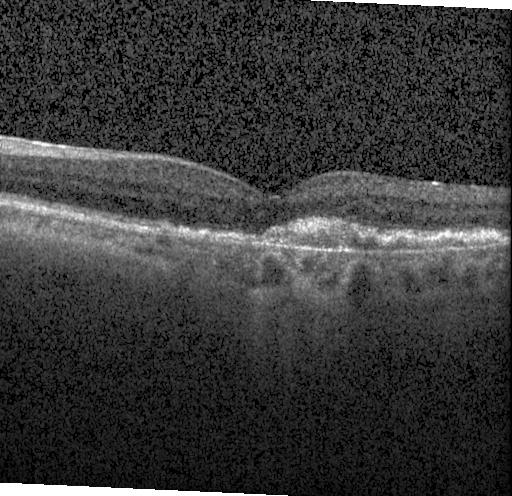

OCT line scan — Diagnosis: a choroidal neovascular membrane.